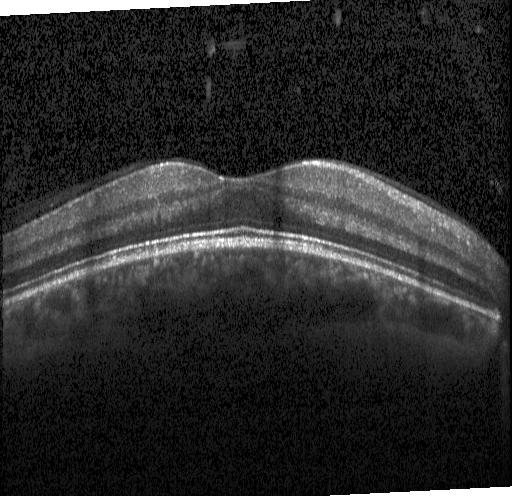 Heidelberg Spectralis, spectral-domain OCT, retinal OCT B-scan. Impression: no choroidal neovascularization, diabetic macular edema, or drusen.